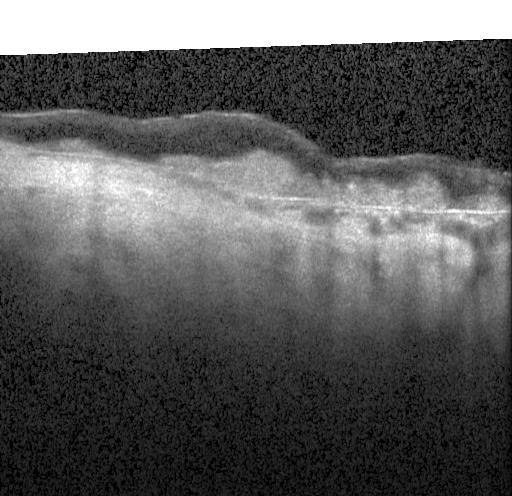

Horizontal scan through the fovea; spectral-domain optical coherence tomography; acquired on a Heidelberg Spectralis; retinal OCT B-scan
Macular OCT: a choroidal neovascular membrane.